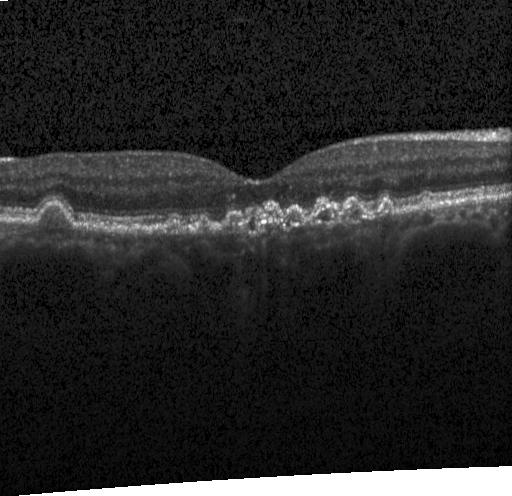

OCT B-scan showing a choroidal neovascular membrane.